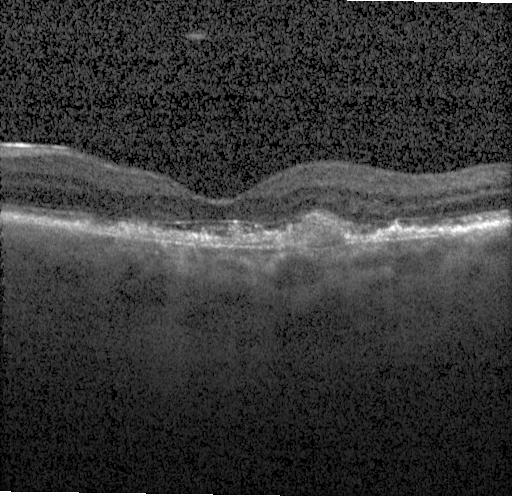
Diagnosis: choroidal neovascularization.